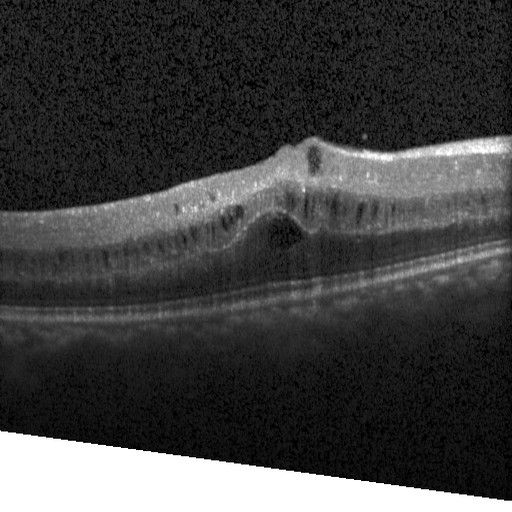 Horizontal scan through the fovea; optical coherence tomography B-scan.
Impression: DME.